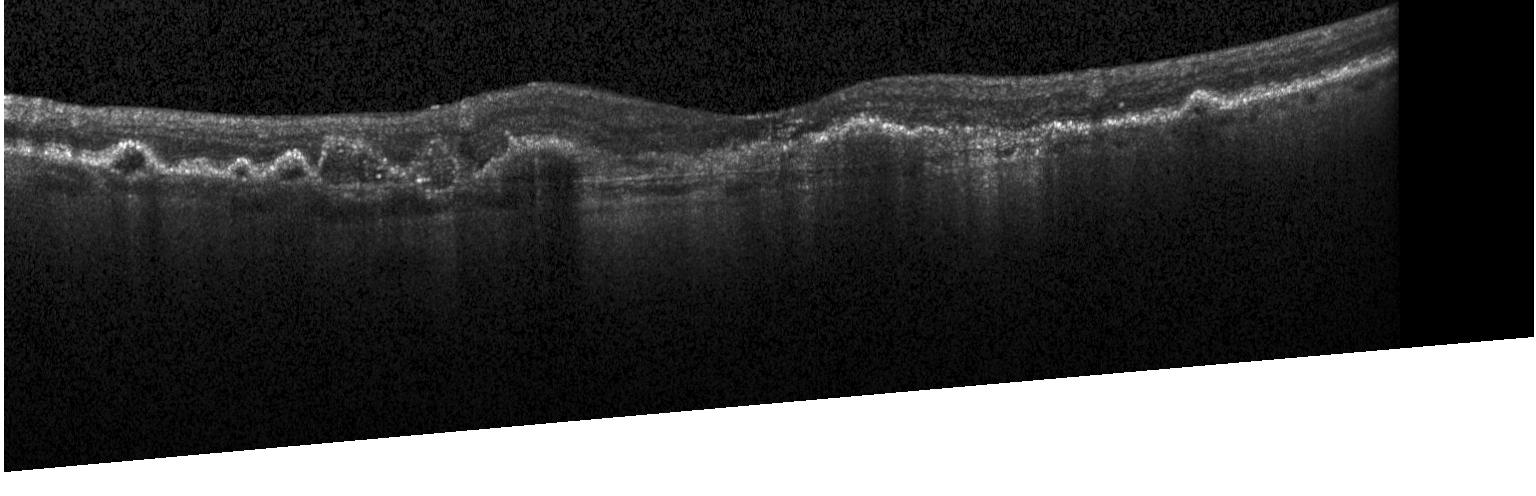 Dx: a choroidal neovascular membrane.